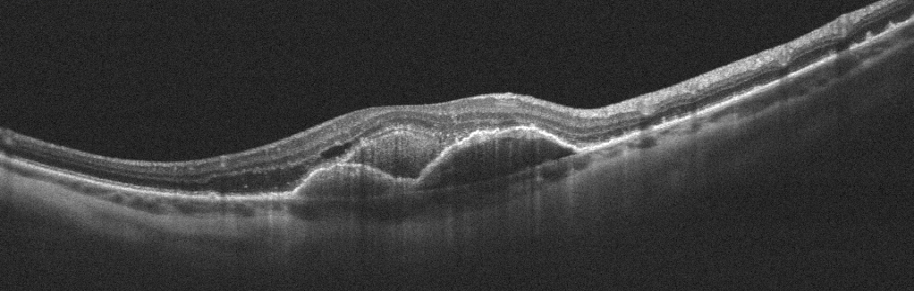

Retinal OCT B-scan, left eye
Impression: AMD.